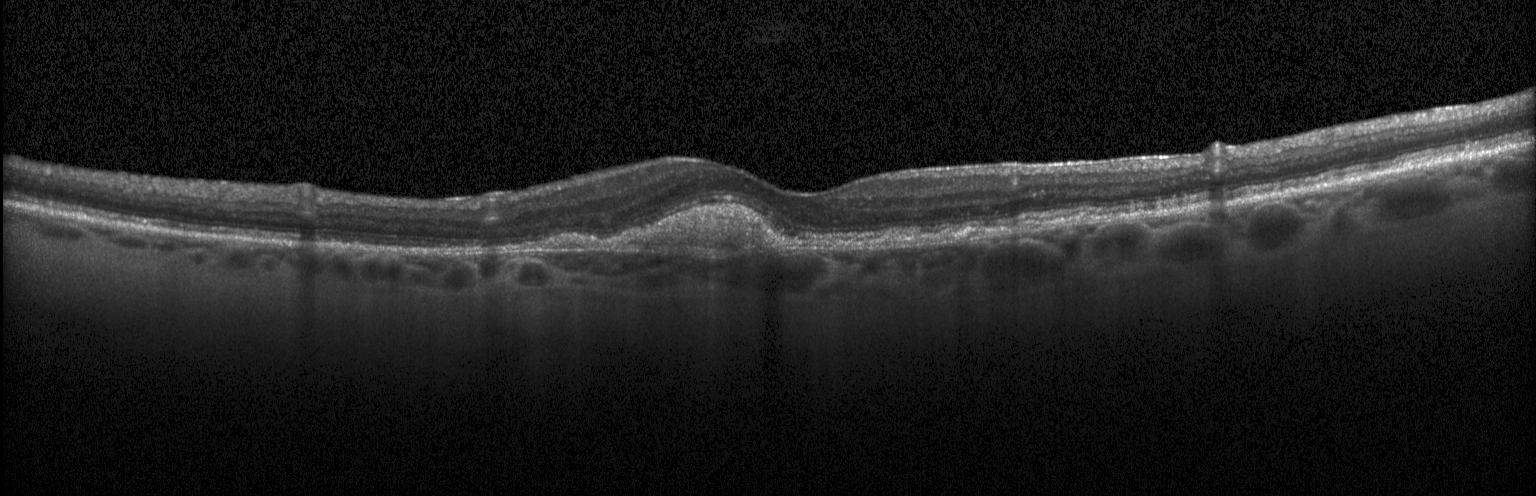

Macular OCT: choroidal neovascularization.